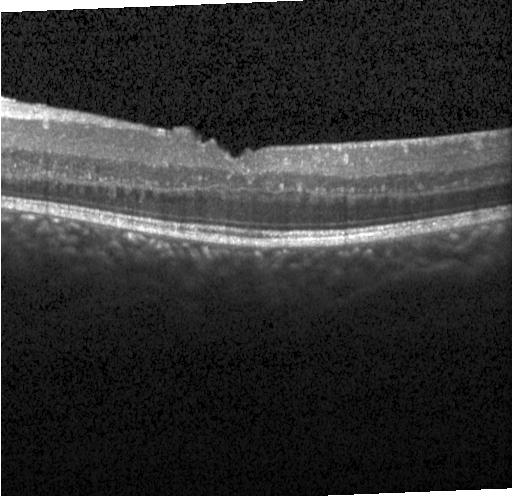

Instrument: Heidelberg Spectralis, spectral-domain OCT, retinal OCT cross-section, macular scan
Finding: diabetic macular edema.